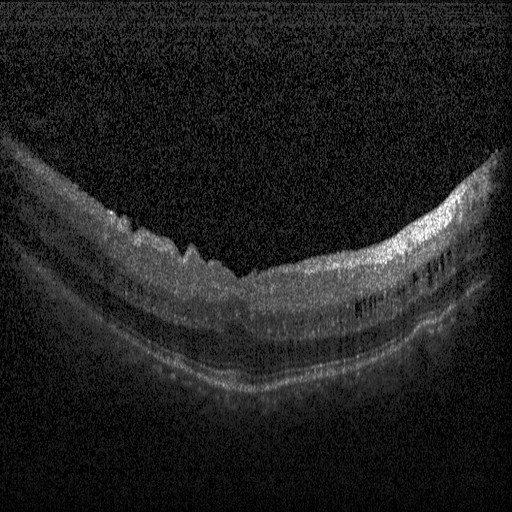 Optical coherence tomography B-scan · through the macula. Finding: diabetic macular edema.